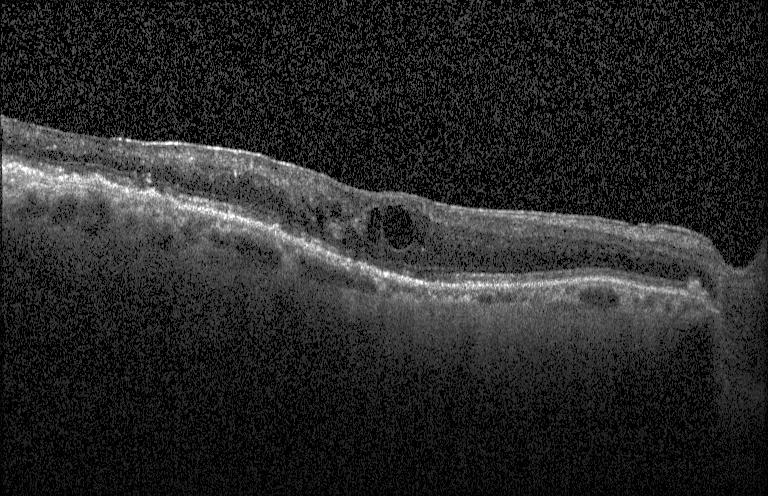

Diagnosis: a choroidal neovascular membrane.